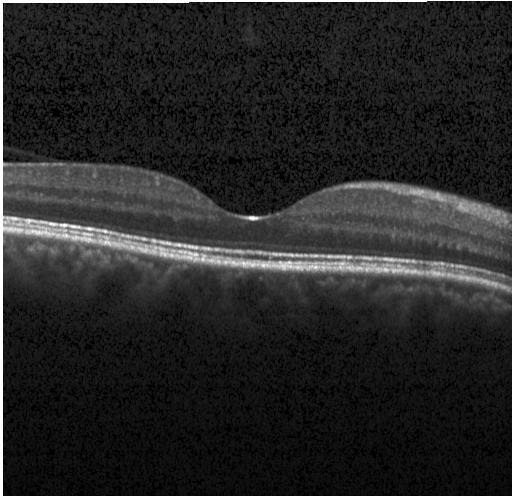

Heidelberg Spectralis. Fovea-centered. OCT B-scan.
OCT finding: neither choroidal neovascularization, diabetic macular edema, nor drusen.